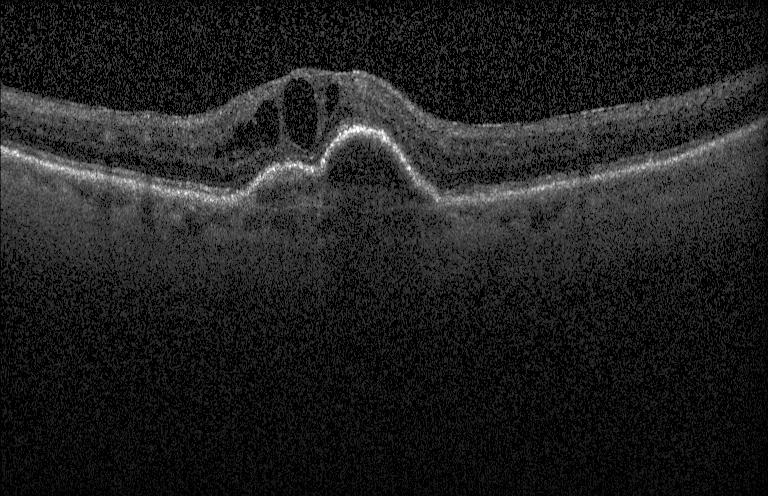

Optical coherence tomography scan.
The scan shows choroidal neovascularization.